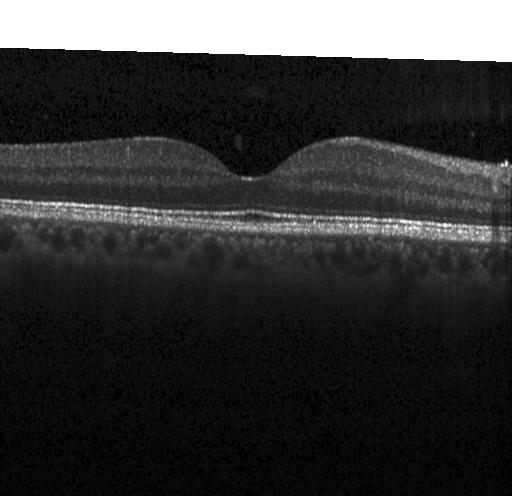 Neither CNV, DME, nor drusen.